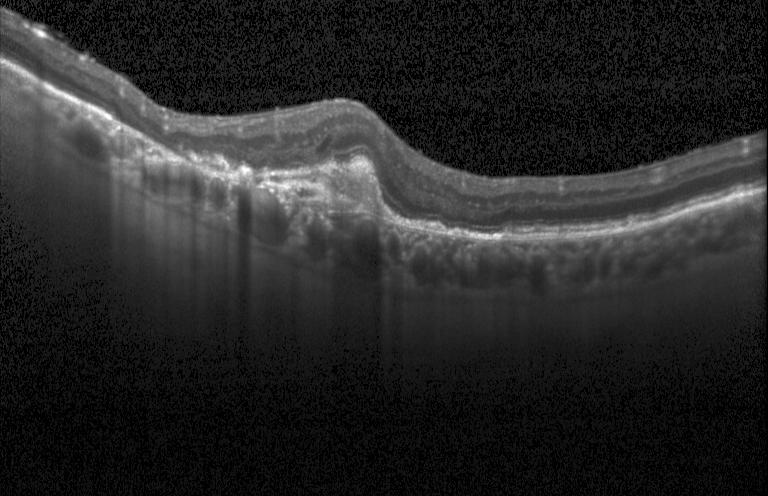 Instrument: Heidelberg Spectralis. Optical coherence tomography scan. Fovea-centered
OCT finding: a choroidal neovascular membrane.